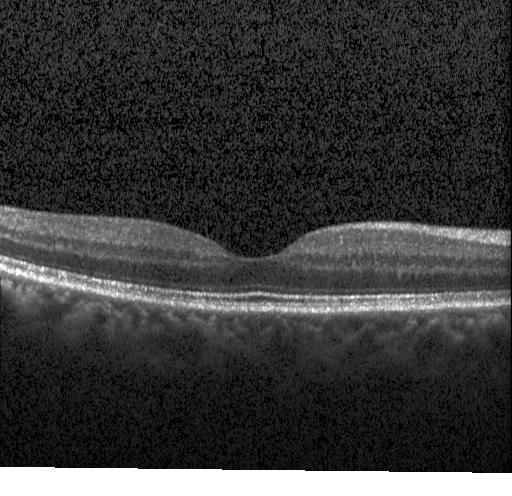

Spectral-domain OCT, Heidelberg Spectralis OCT system, macular scan, OCT line scan — Assessment: no evidence of CNV, DME, or drusen.